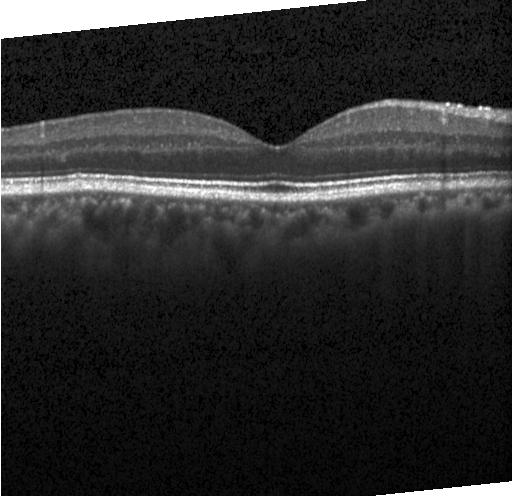 The scan shows no choroidal neovascularization, diabetic macular edema, or drusen.